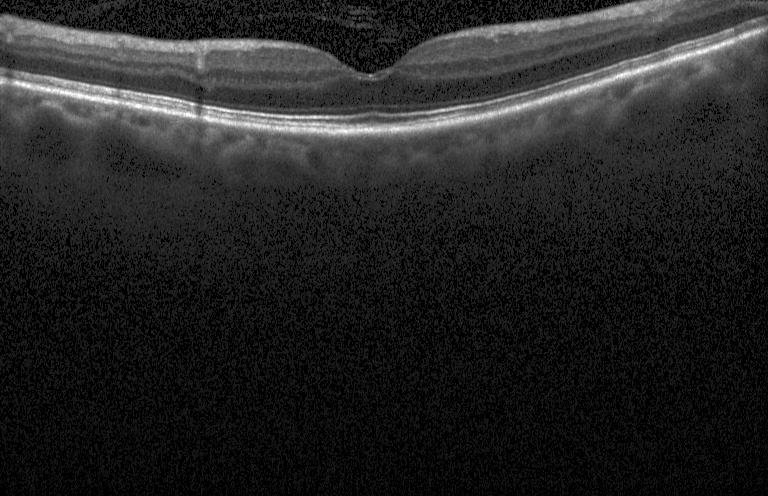

Macular OCT: neither choroidal neovascularization, diabetic macular edema, nor drusen.